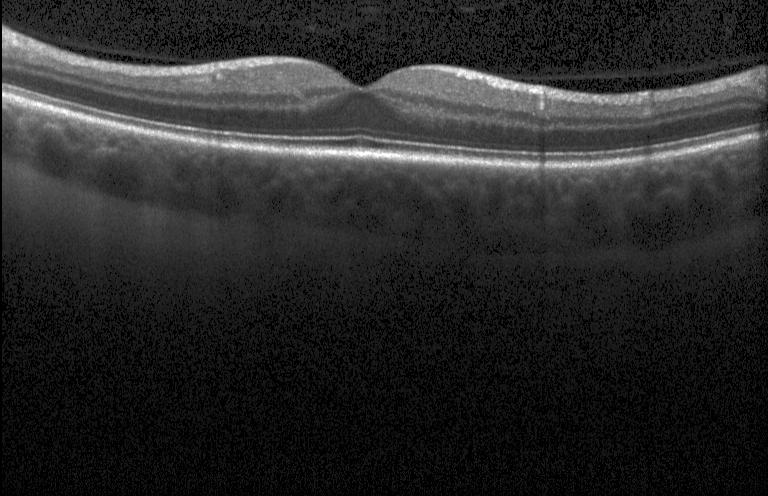

OCT line scan, centered on the fovea.
This B-scan demonstrates no choroidal neovascularization, diabetic macular edema, or drusen.